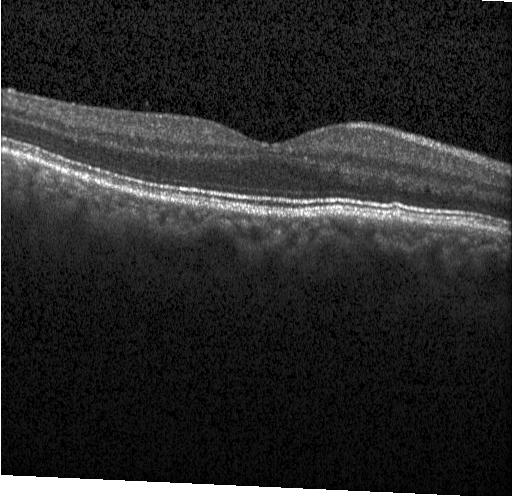

Impression: no choroidal neovascularization, diabetic macular edema, or drusen.